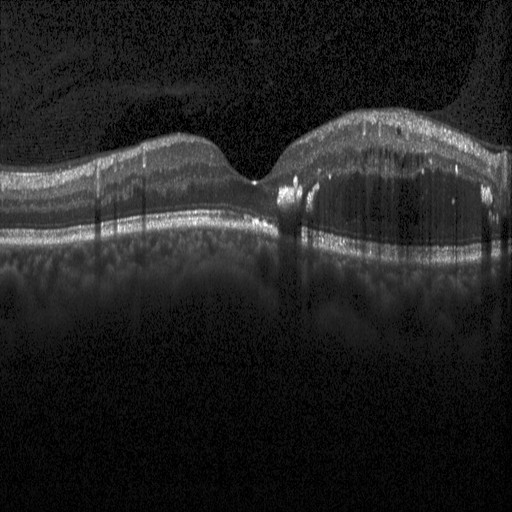

The scan shows DME.